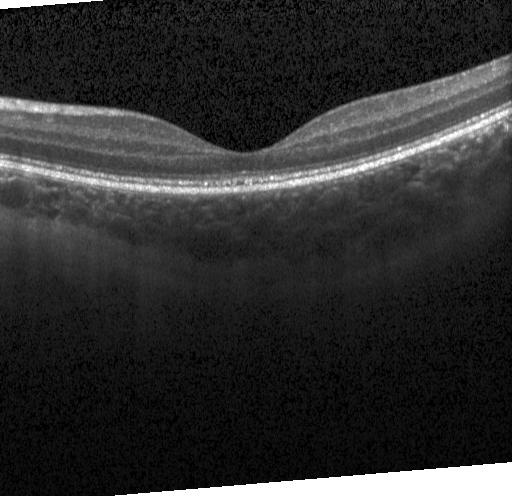 Heidelberg Spectralis OCT system. OCT B-scan. Fovea-centered.
Finding: neither choroidal neovascularization, diabetic macular edema, nor drusen.